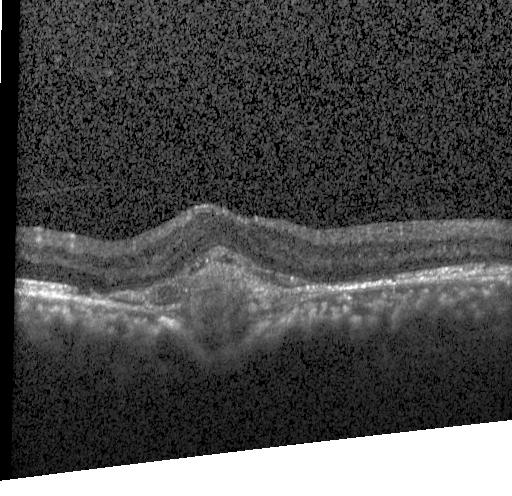 Impression: a choroidal neovascular membrane.